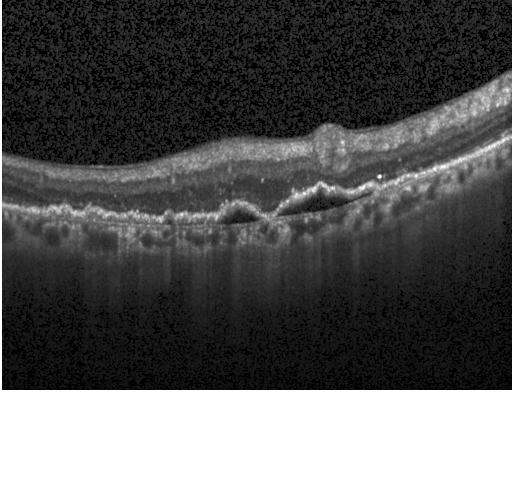
Impression: choroidal neovascularization.